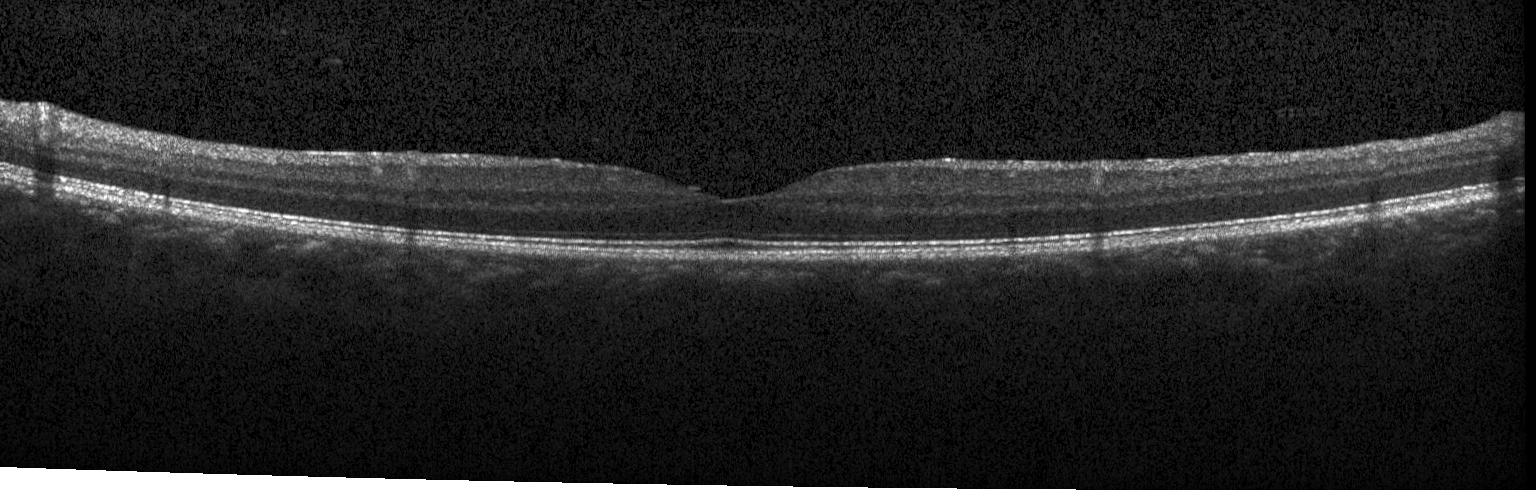 Optical coherence tomography B-scan. Acquired on a Heidelberg Spectralis
Macular OCT: neither CNV, DME, nor drusen.